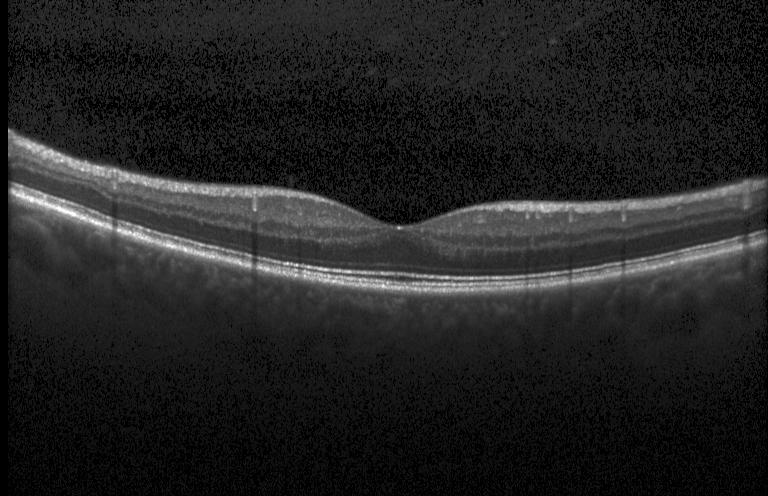
Optical coherence tomography scan; SD-OCT. OCT finding: neither choroidal neovascularization, diabetic macular edema, nor drusen.